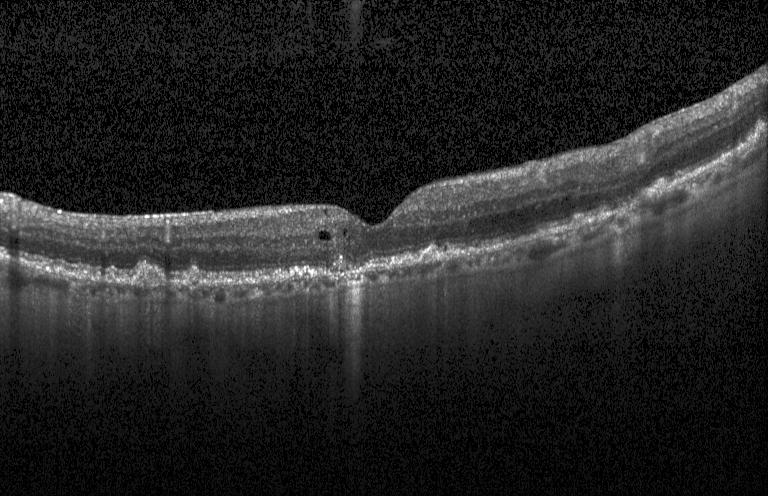 Spectral-domain OCT; fovea-centered; Heidelberg Spectralis; optical coherence tomography B-scan.
Impression: a choroidal neovascular membrane.